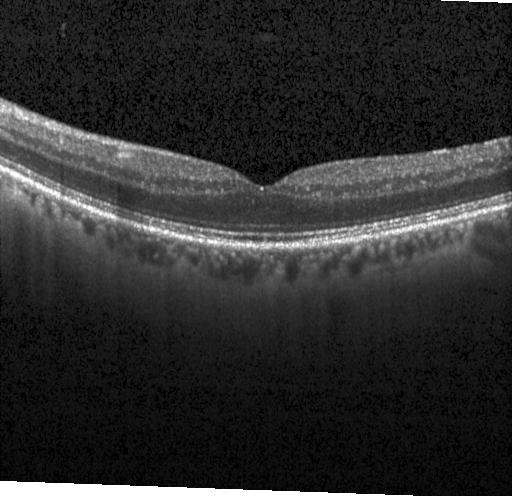 Retinal OCT cross-section.
Finding: neither choroidal neovascularization, diabetic macular edema, nor drusen.